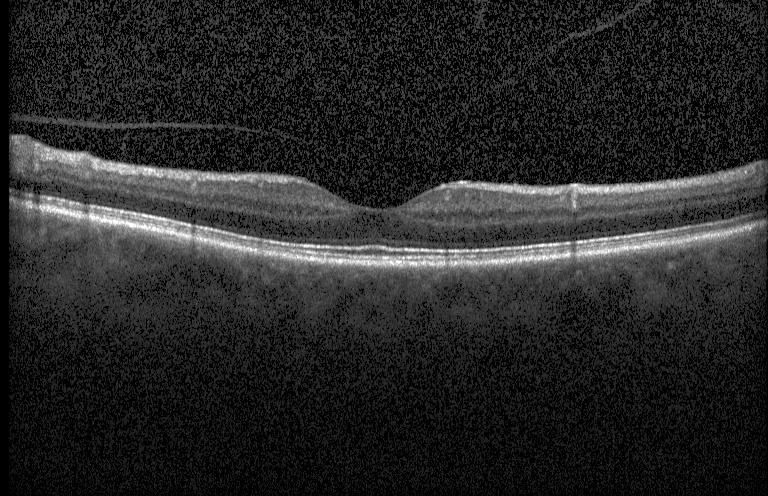 Retinal OCT B-scan.
Finding: no choroidal neovascularization, diabetic macular edema, or drusen.